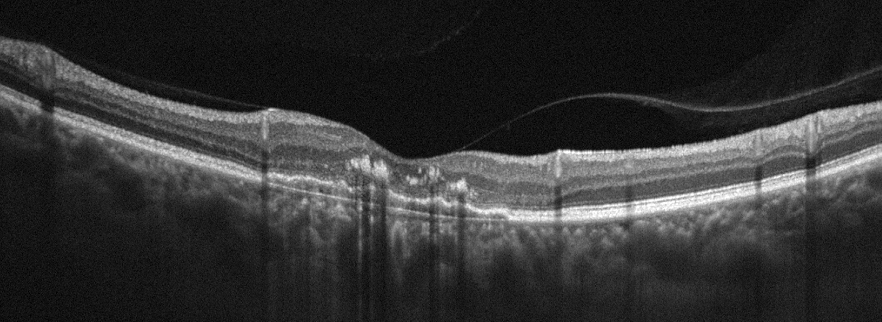 OS. Retinal OCT B-scan
Impression: age-related macular degeneration.